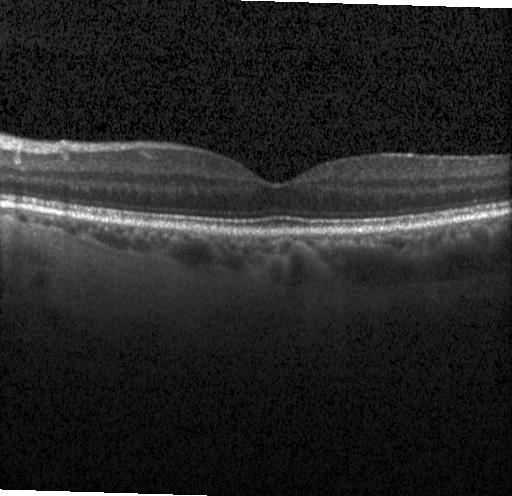
OCT scan showing no choroidal neovascularization, no diabetic macular edema, and no drusen.